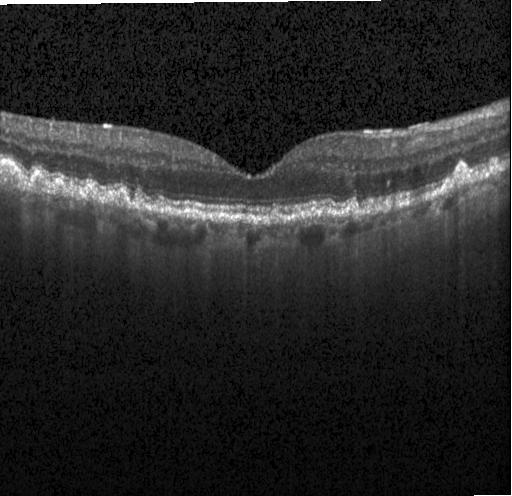 OCT line scan. SD-OCT.
The scan shows multiple drusen.